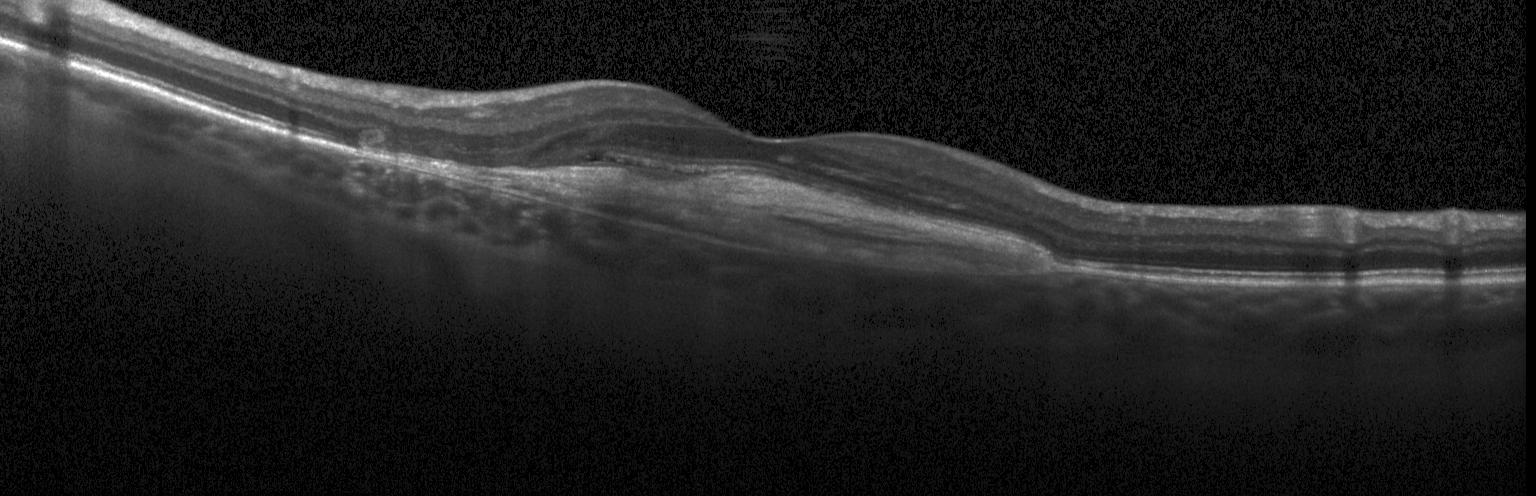 Retinal OCT cross-section. SD-OCT. Fovea-centered.
Finding: CNV.